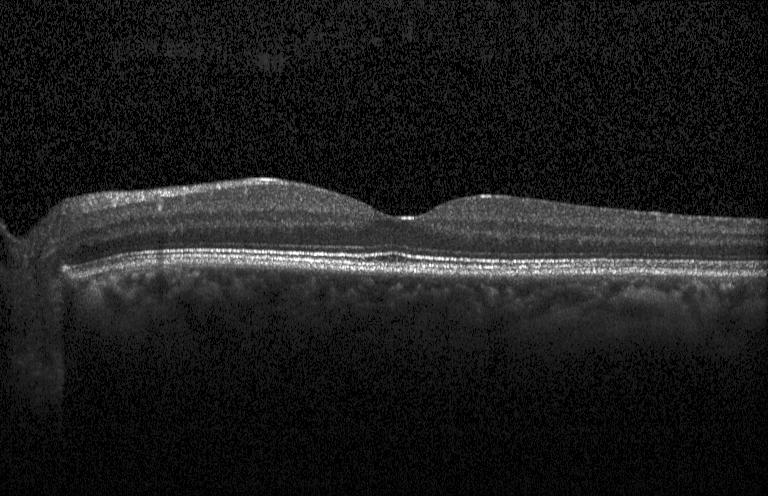
Macular OCT: no choroidal neovascularization, no diabetic macular edema, and no drusen.